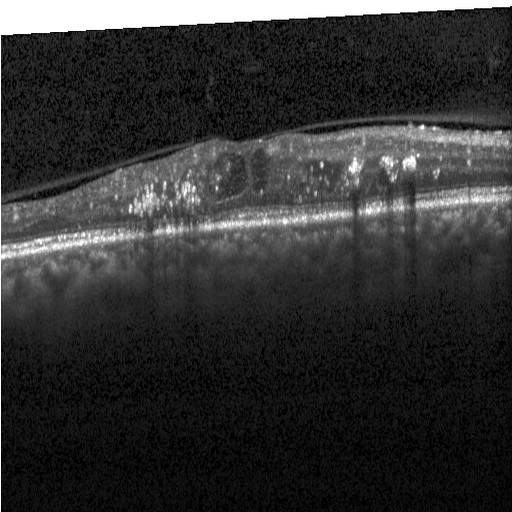

OCT B-scan.
Finding: diabetic macular edema.